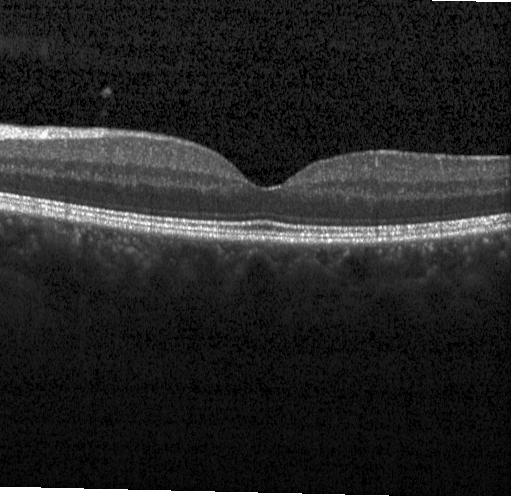

Dx: no evidence of choroidal neovascularization, diabetic macular edema, or drusen.